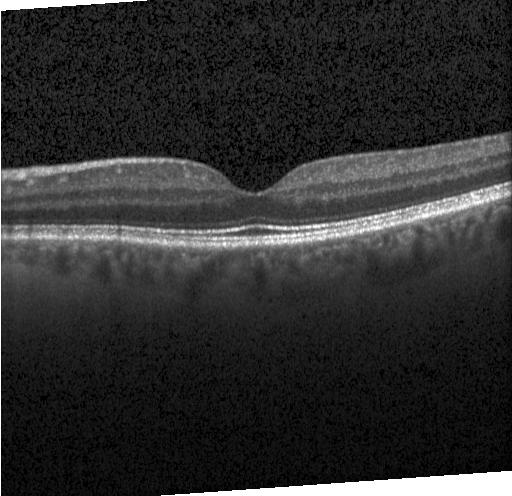

Spectral-domain OCT B-scan: no evidence of choroidal neovascularization, diabetic macular edema, or drusen.